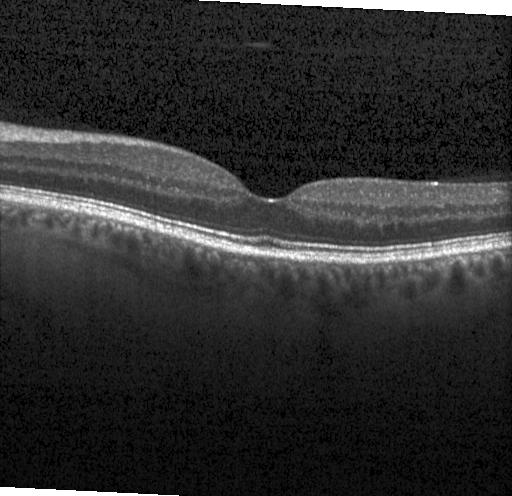

Instrument: Heidelberg Spectralis · horizontal scan through the fovea · retinal OCT cross-section. Dx: no evidence of choroidal neovascularization, diabetic macular edema, or drusen.